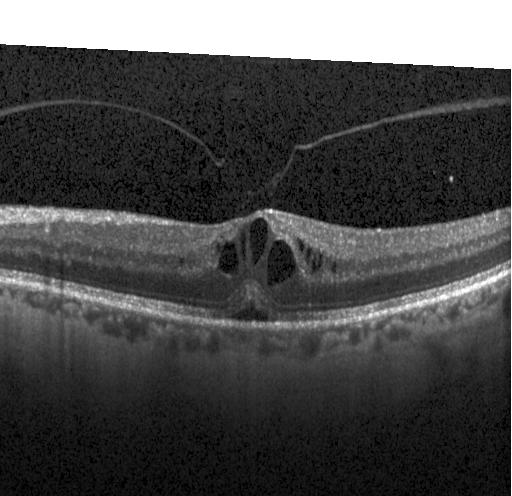
Assessment: diabetic macular edema (DME).